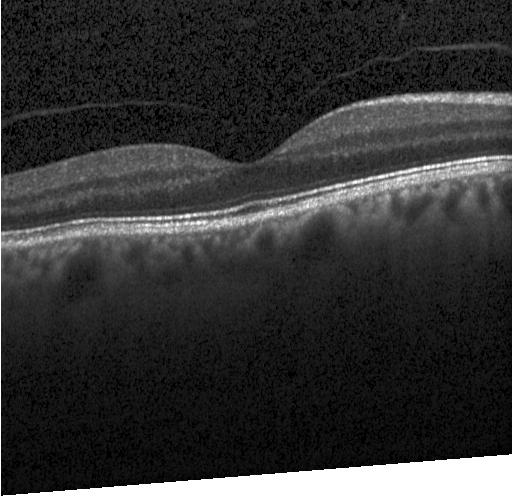
OCT B-scan
OCT finding: no evidence of choroidal neovascularization, diabetic macular edema, or drusen.